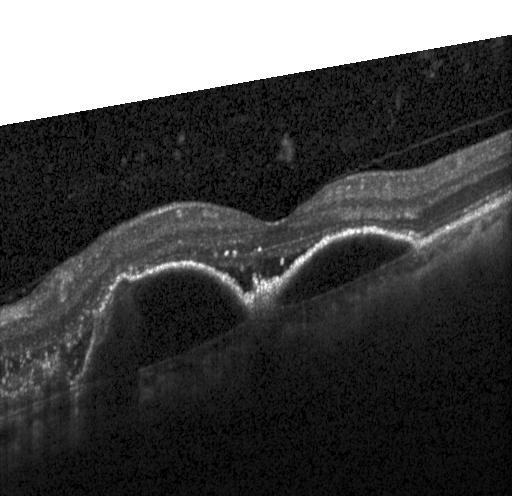

Fovea-centered · optical coherence tomography scan. Dx: a choroidal neovascular membrane.